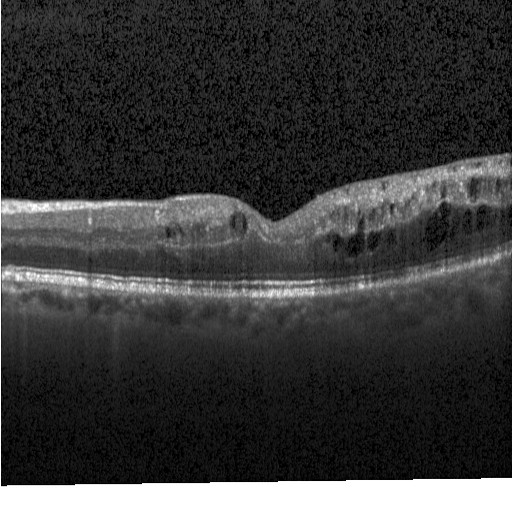

Horizontal scan through the fovea, SD-OCT, OCT line scan
The scan shows diabetic macular edema.